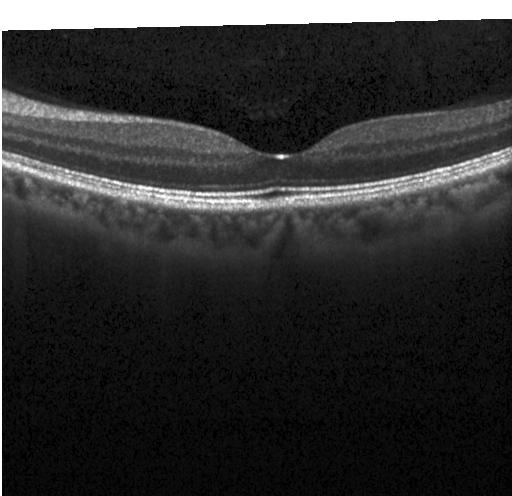
Heidelberg Spectralis, spectral-domain optical coherence tomography, fovea-centered, retinal OCT cross-section.
This B-scan demonstrates no choroidal neovascularization, no diabetic macular edema, and no drusen.